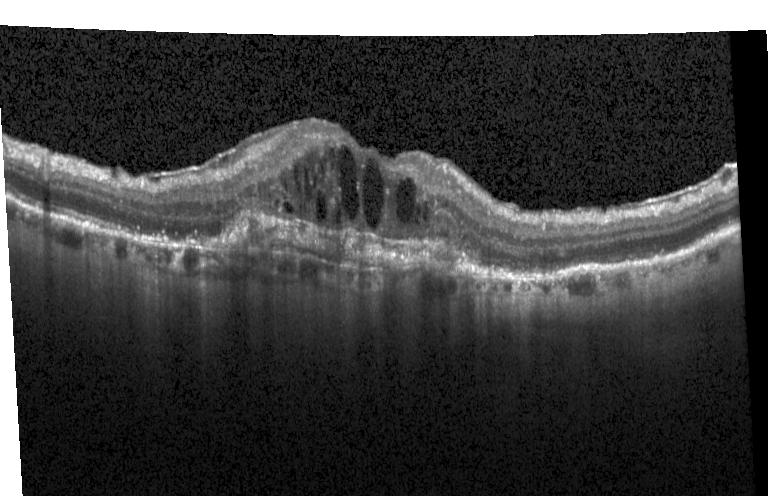 Macular OCT demonstrating choroidal neovascularization.